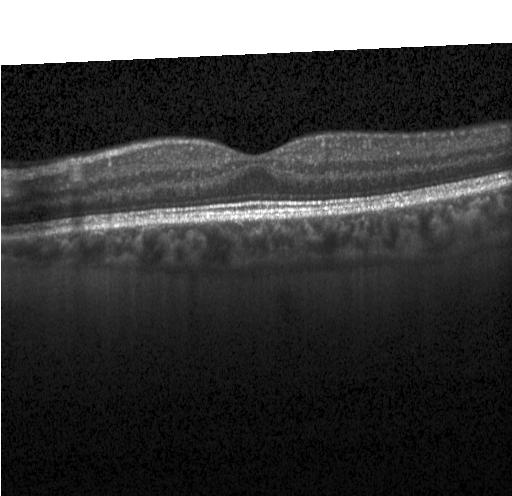 Finding: no CNV, DME, or drusen.